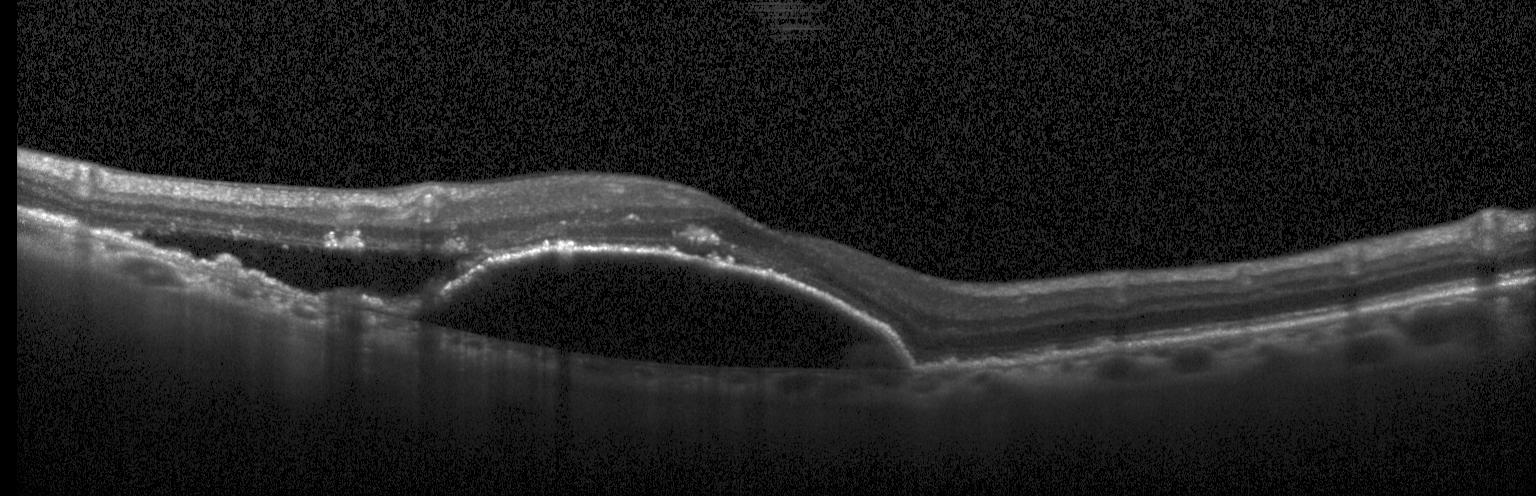

Impression: CNV.